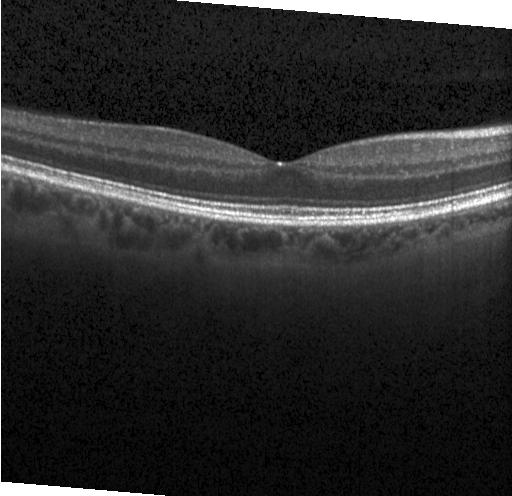 Macular OCT demonstrating neither choroidal neovascularization, diabetic macular edema, nor drusen.